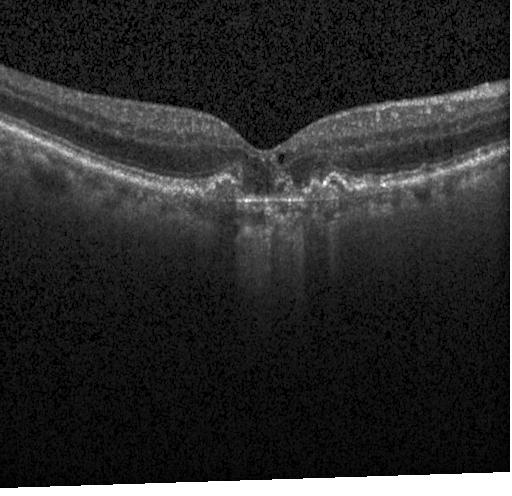
Spectral-domain optical coherence tomography. Macular scan. Optical coherence tomography scan. Heidelberg Spectralis. This B-scan demonstrates a choroidal neovascular membrane.